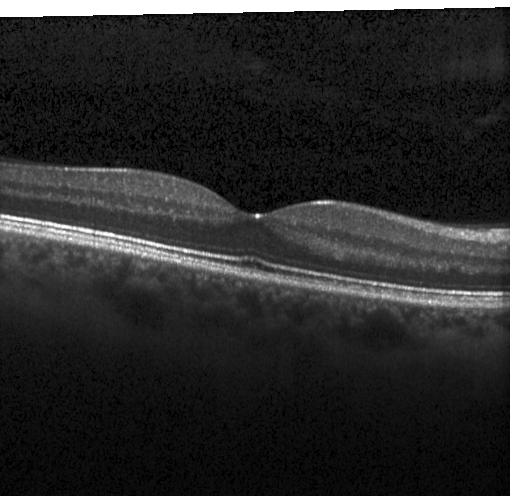

Spectral-domain OCT B-scan: no choroidal neovascularization, no diabetic macular edema, and no drusen.